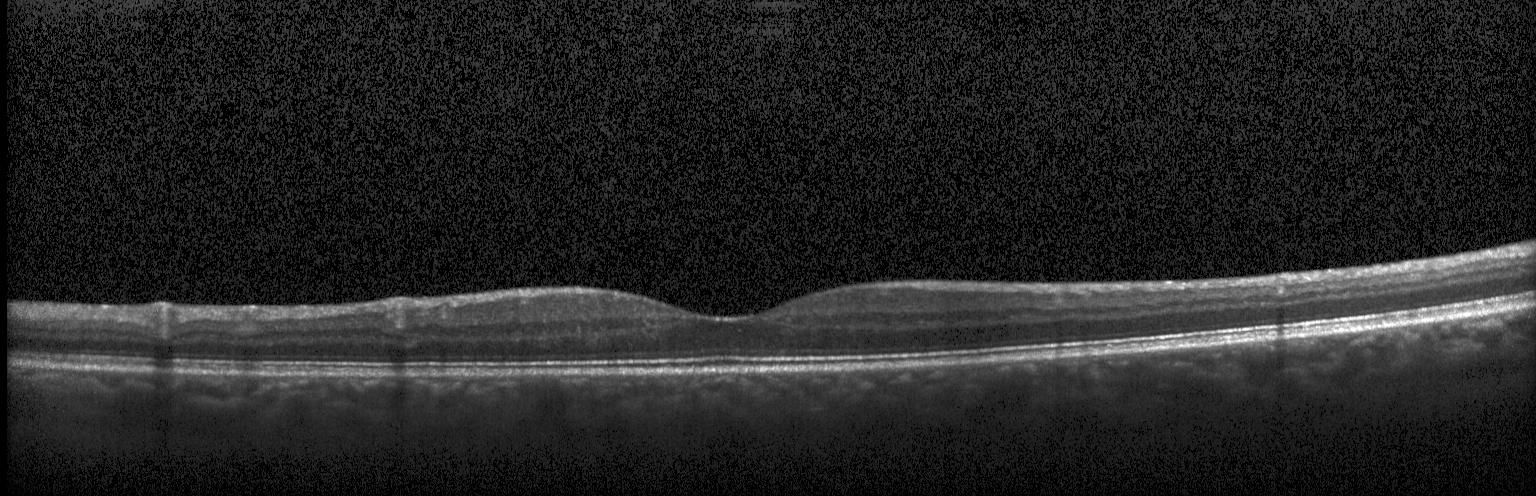

Horizontal scan through the fovea, instrument: Heidelberg Spectralis, retinal OCT cross-section, SD-OCT — This B-scan demonstrates no choroidal neovascularization, no diabetic macular edema, and no drusen.